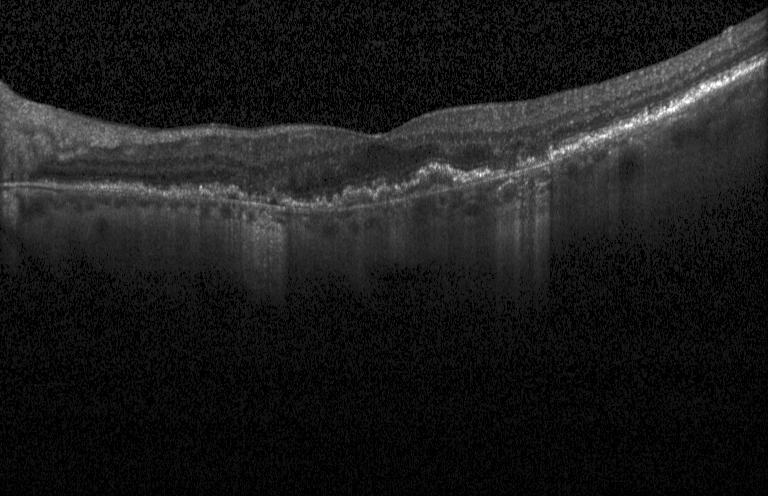

Impression: a choroidal neovascular membrane.